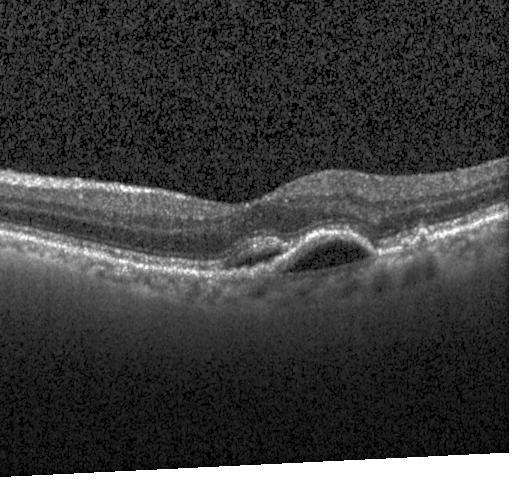 Macular OCT demonstrating CNV.